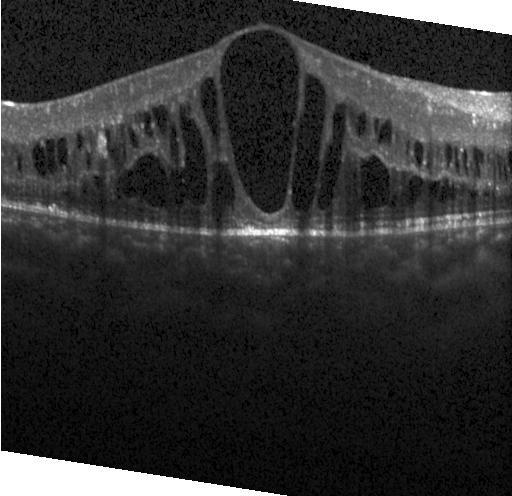 Spectral-domain OCT B-scan: diabetic macular edema (DME).